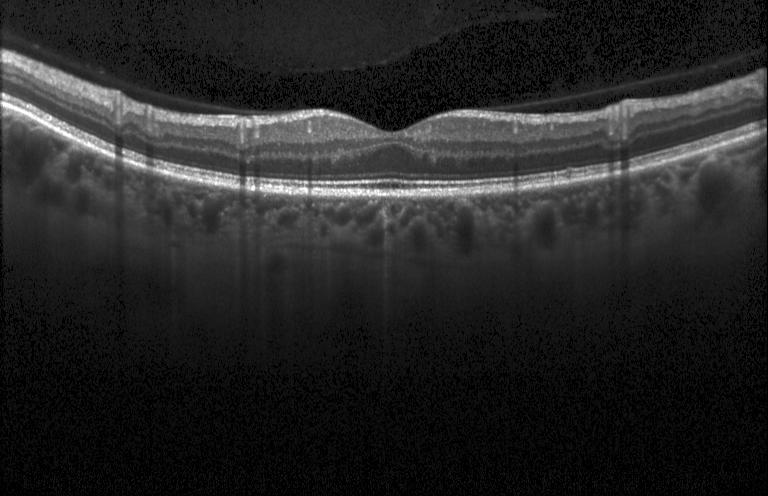
SD-OCT. Heidelberg Spectralis. Macular scan. Optical coherence tomography scan — Finding: no evidence of CNV, DME, or drusen.